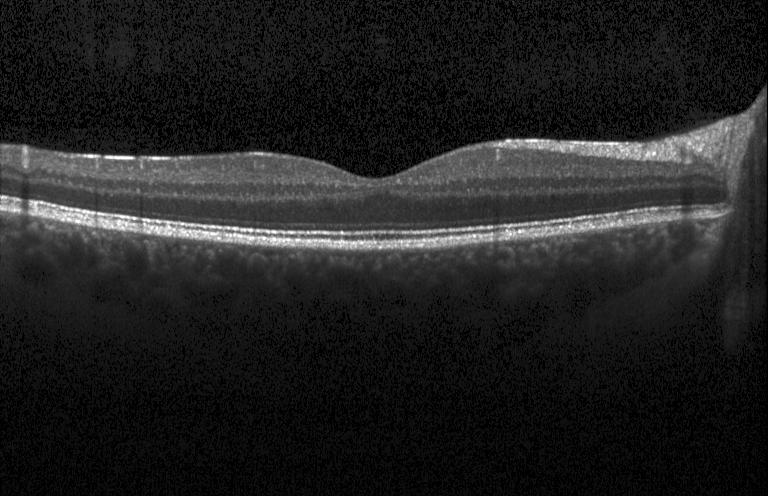 Macular OCT: no choroidal neovascularization, diabetic macular edema, or drusen.